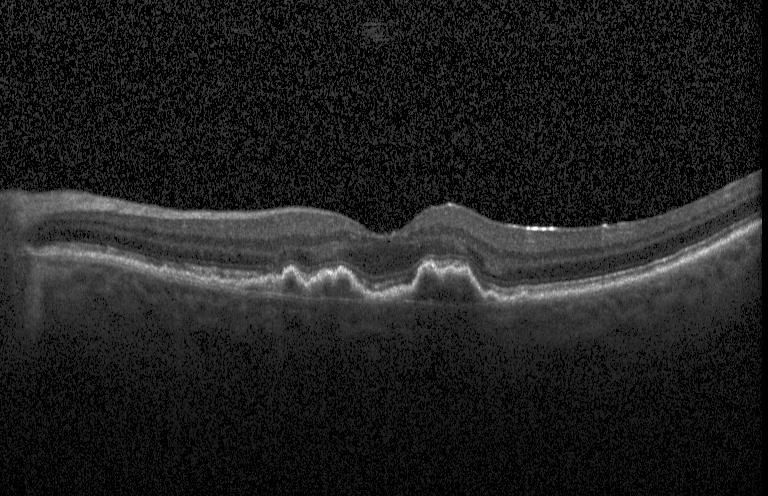
Optical coherence tomography B-scan
The scan shows a choroidal neovascular membrane.